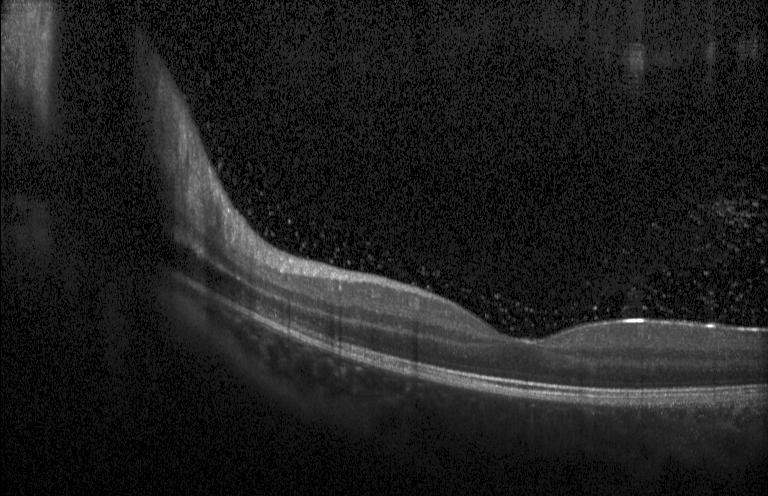

Heidelberg Spectralis · OCT line scan
Finding: neither CNV, DME, nor drusen.